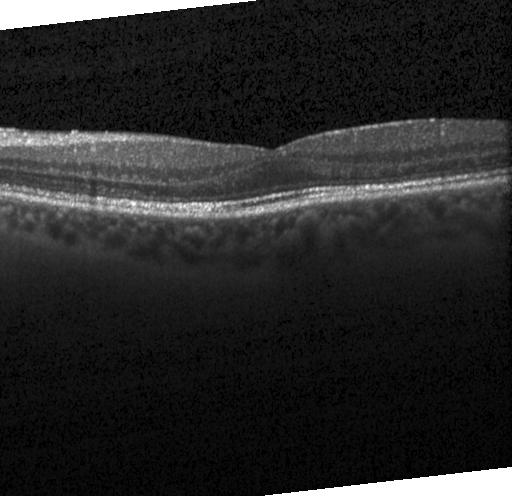

OCT scan showing no evidence of CNV, DME, or drusen.